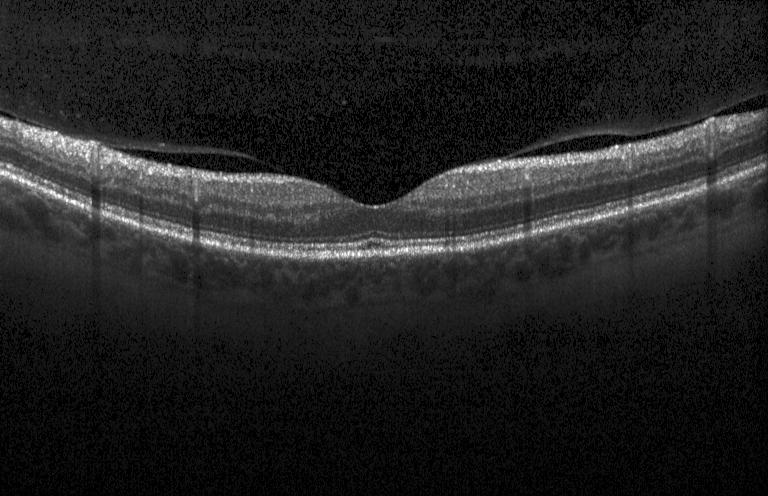
Retinal OCT B-scan. Spectral-domain OCT — OCT finding: no evidence of choroidal neovascularization, diabetic macular edema, or drusen.